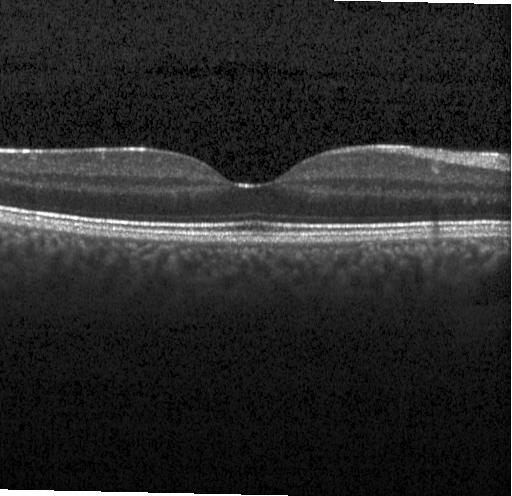

Spectral-domain optical coherence tomography · fovea-centered · retinal OCT cross-section · instrument: Heidelberg Spectralis. Neither CNV, DME, nor drusen.